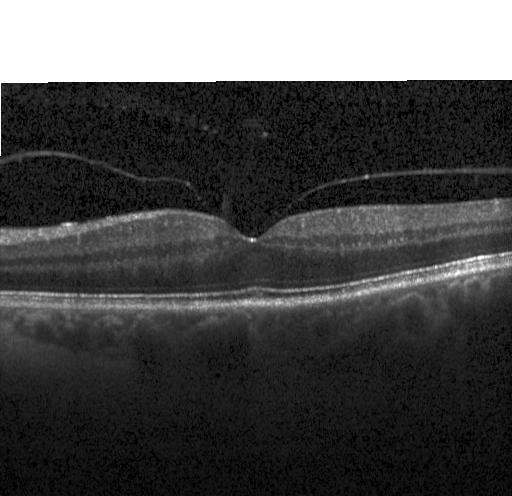 OCT B-scan, SD-OCT, instrument: Heidelberg Spectralis
Diagnosis: no choroidal neovascularization, diabetic macular edema, or drusen.